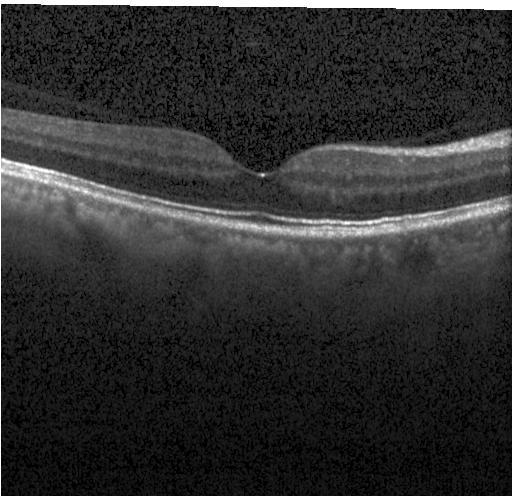
The scan shows no choroidal neovascularization, no diabetic macular edema, and no drusen.